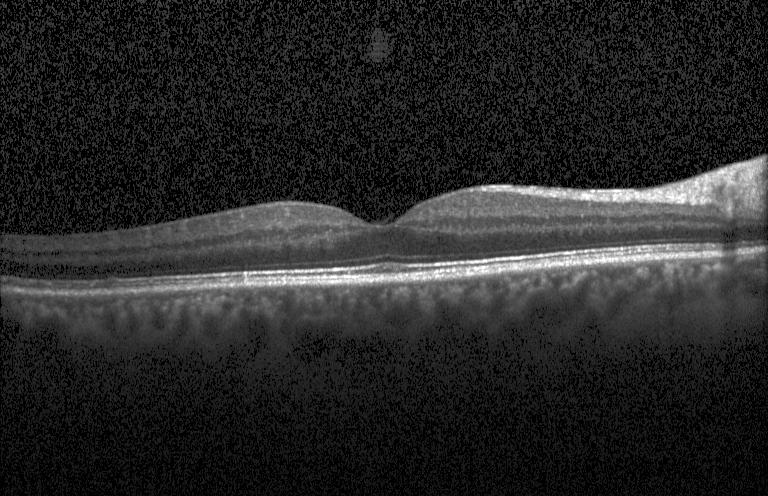
Optical coherence tomography scan · acquired on a Heidelberg Spectralis — Diagnosis: neither choroidal neovascularization, diabetic macular edema, nor drusen.